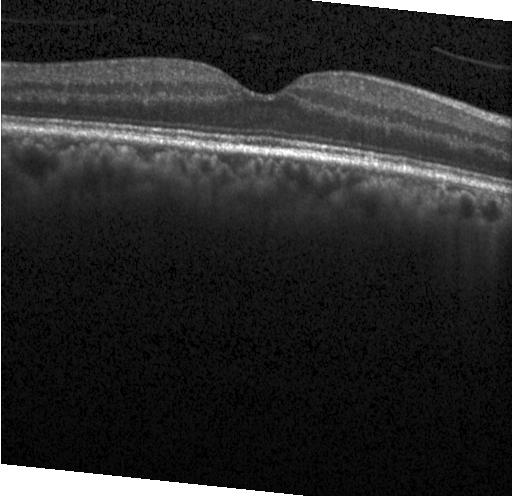
OCT B-scan. SD-OCT.
Dx: no choroidal neovascularization, diabetic macular edema, or drusen.